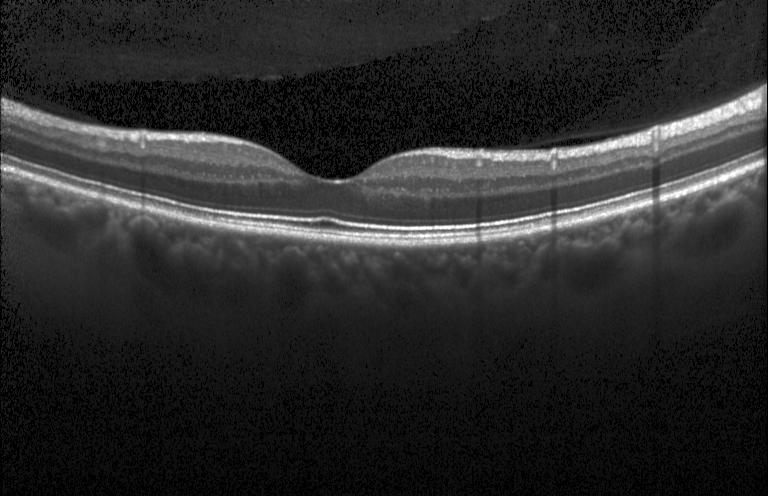
The scan shows no evidence of CNV, DME, or drusen.